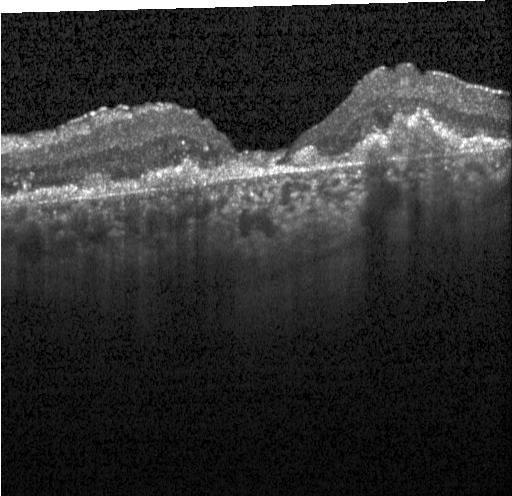
Retinal OCT cross-section
Impression: a choroidal neovascular membrane.